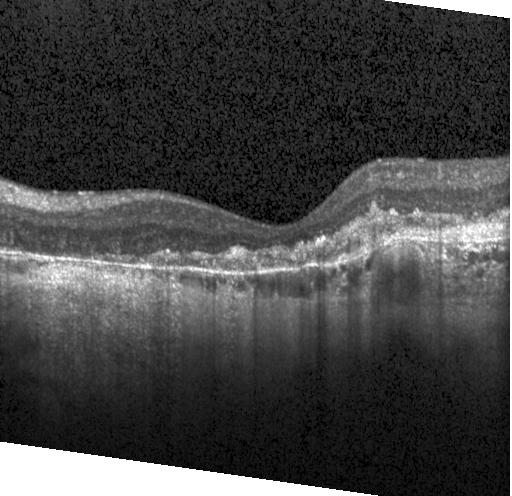 Macular OCT: CNV.